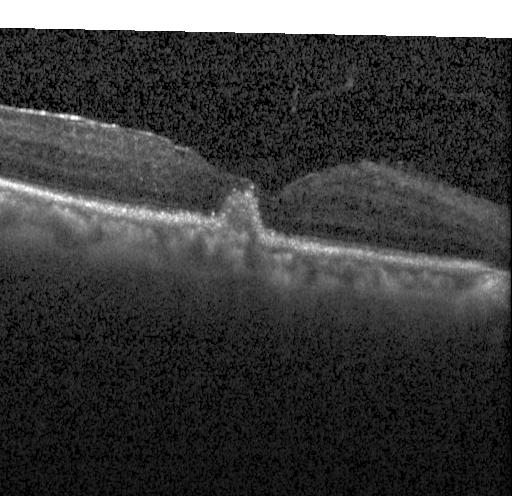
Spectral-domain optical coherence tomography · horizontal scan through the fovea · optical coherence tomography B-scan — Diagnosis: a choroidal neovascular membrane.